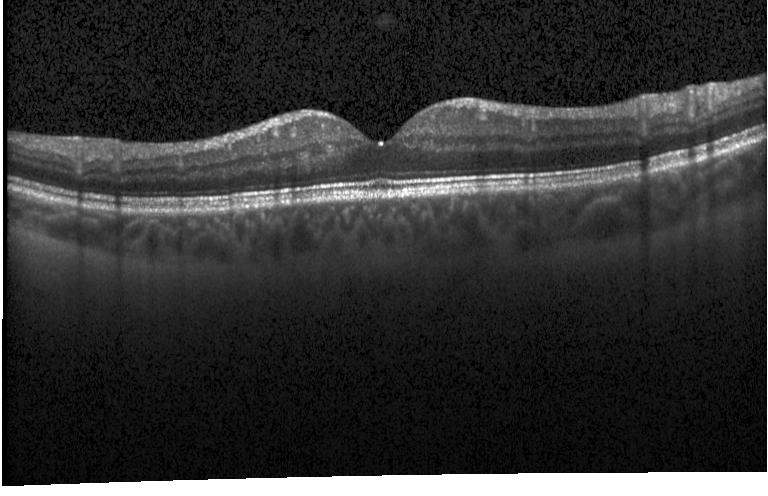

Retinal OCT B-scan
Finding: no CNV, no DME, and no drusen.